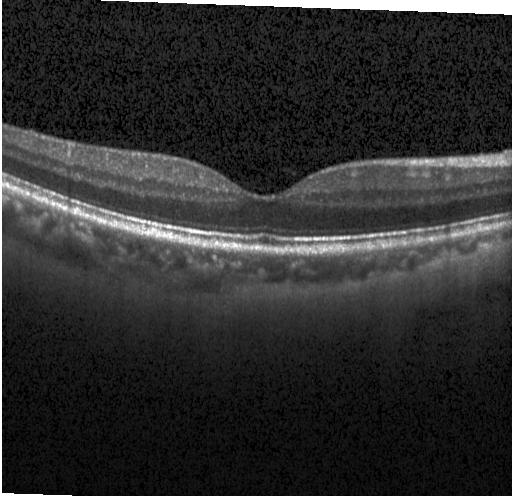 Optical coherence tomography B-scan.
Macular OCT: neither CNV, DME, nor drusen.